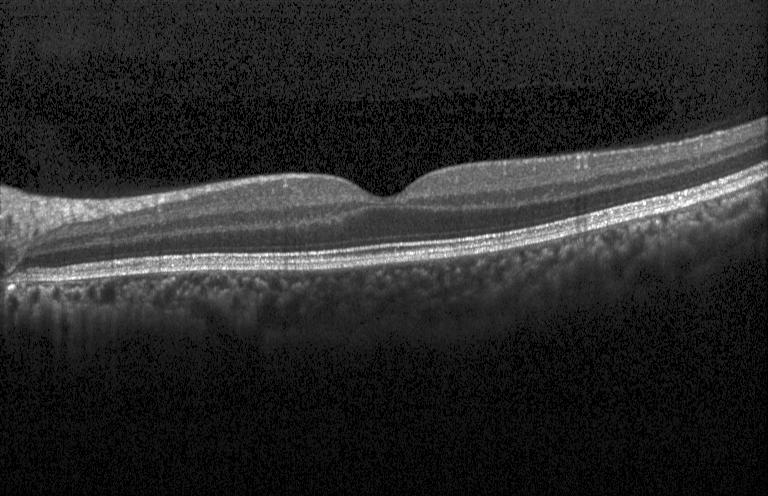

Fovea-centered · instrument: Heidelberg Spectralis · spectral-domain optical coherence tomography · retinal OCT cross-section
OCT finding: no evidence of CNV, DME, or drusen.